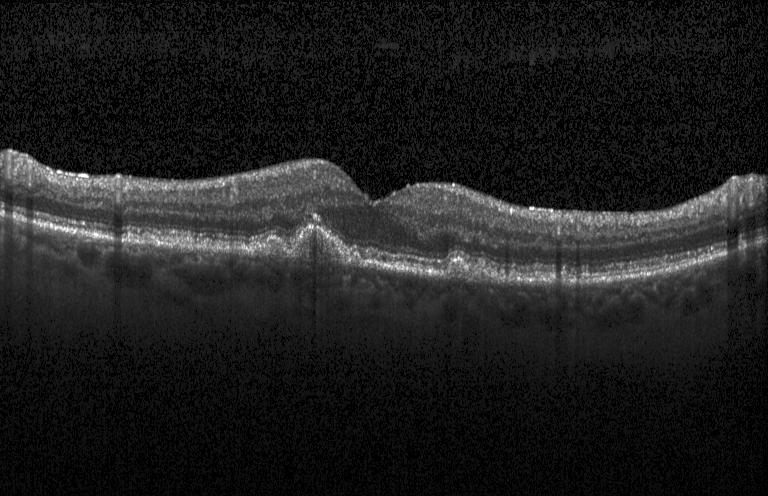 Spectral-domain OCT B-scan: sub-RPE drusenoid deposits.